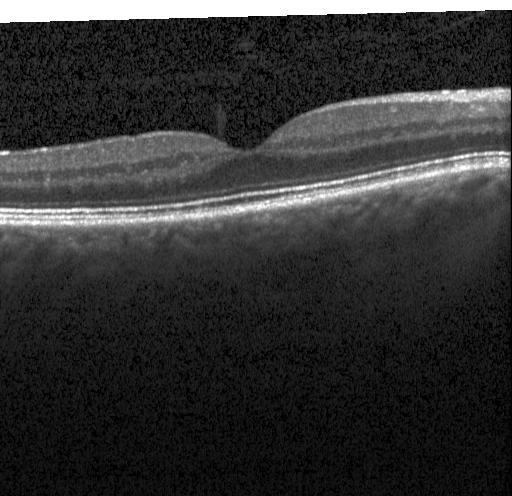 OCT line scan — Finding: no evidence of CNV, DME, or drusen.